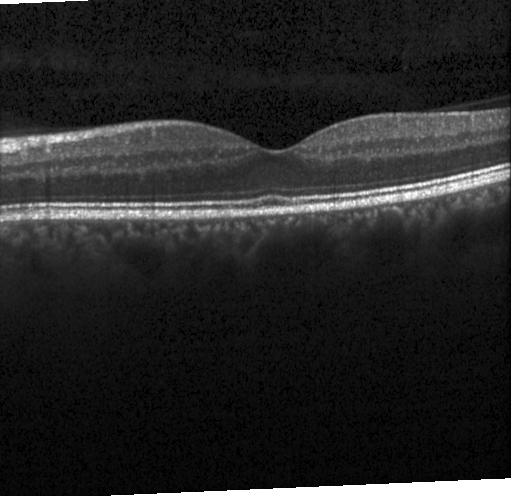 Spectral-domain OCT; retinal OCT cross-section; instrument: Heidelberg Spectralis
Dx: neither choroidal neovascularization, diabetic macular edema, nor drusen.